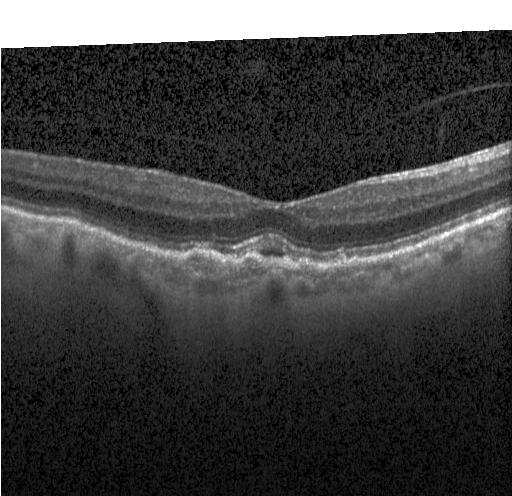

Horizontal scan through the fovea · OCT B-scan · instrument: Heidelberg Spectralis · spectral-domain optical coherence tomography.
OCT finding: a choroidal neovascular membrane.